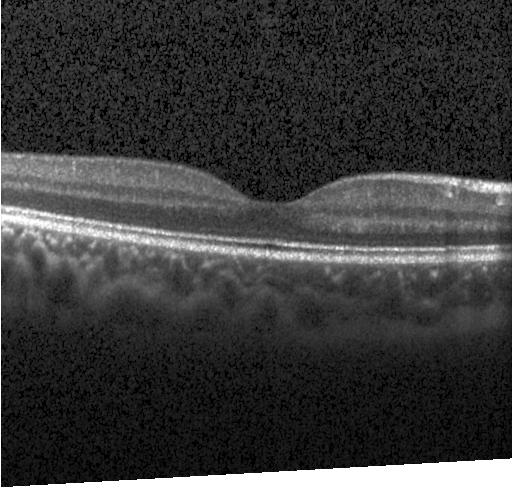 OCT line scan.
Impression: no CNV, no DME, and no drusen.